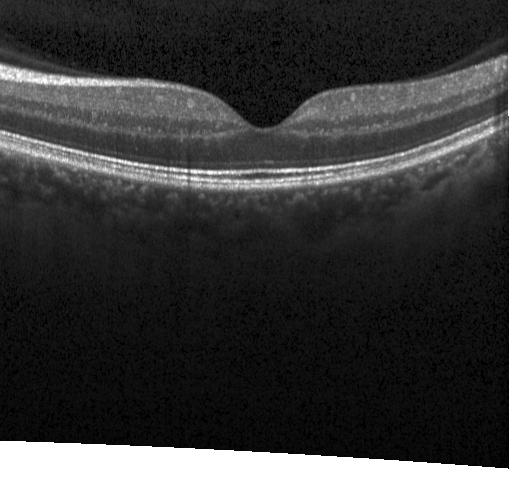 Instrument: Heidelberg Spectralis. Horizontal scan through the fovea. Spectral-domain OCT. Optical coherence tomography scan — Finding: no choroidal neovascularization, no diabetic macular edema, and no drusen.